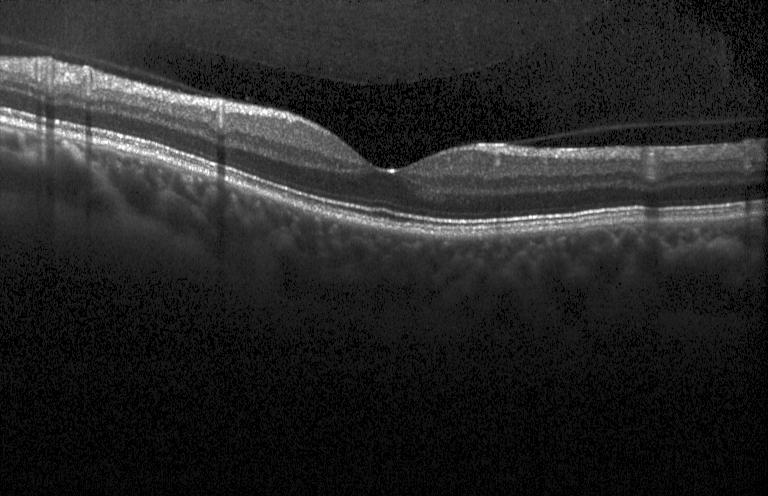
Instrument: Heidelberg Spectralis · fovea-centered · optical coherence tomography B-scan — Finding: neither CNV, DME, nor drusen.